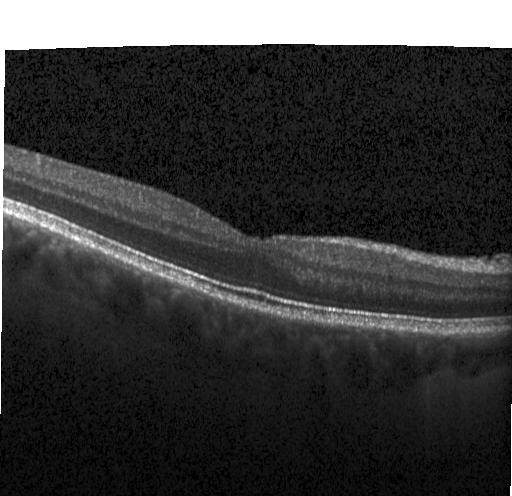
Optical coherence tomography scan. Centered on the fovea
Impression: no evidence of choroidal neovascularization, diabetic macular edema, or drusen.